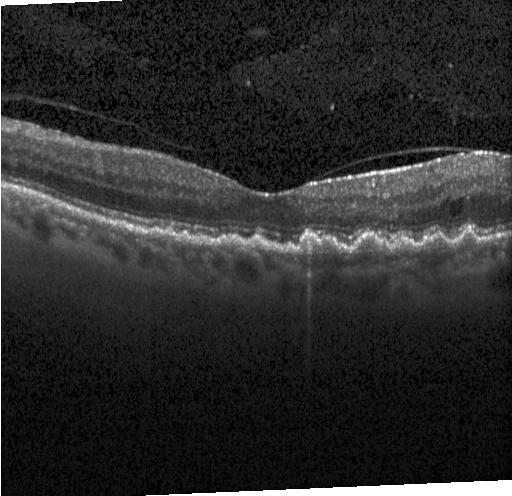
Macular scan, OCT B-scan, Heidelberg Spectralis OCT system. Dx: a choroidal neovascular membrane.